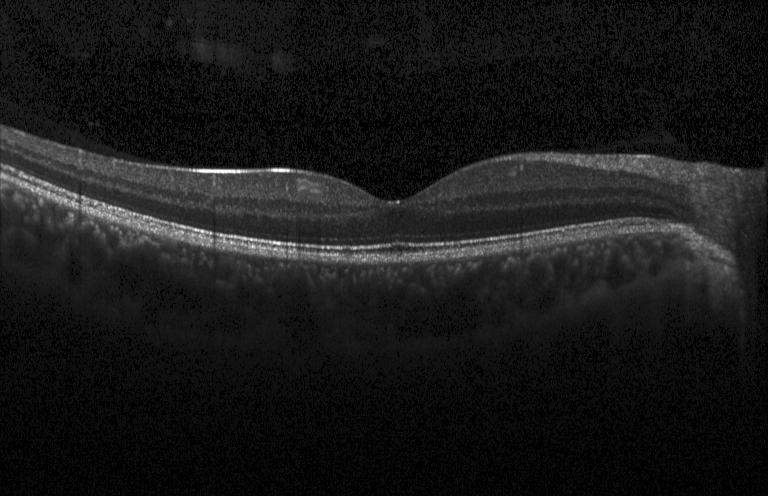 Optical coherence tomography scan; spectral-domain OCT. Impression: no choroidal neovascularization, diabetic macular edema, or drusen.